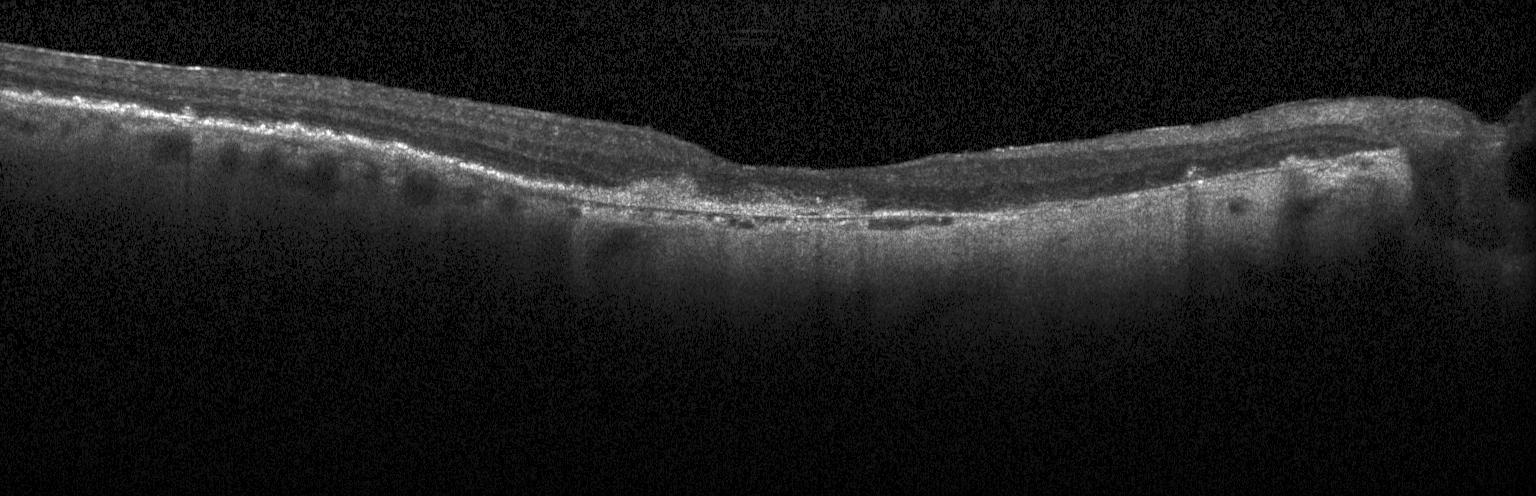
Acquired on a Heidelberg Spectralis. Through the macula. Optical coherence tomography scan — The scan shows choroidal neovascularization (CNV).